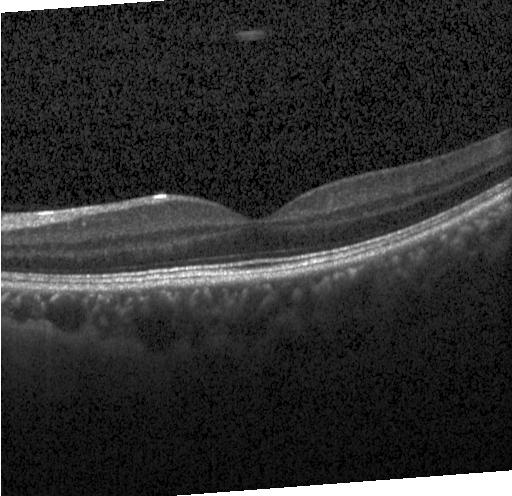 OCT B-scan. Spectral-domain optical coherence tomography. Macular scan. OCT finding: no evidence of choroidal neovascularization, diabetic macular edema, or drusen.